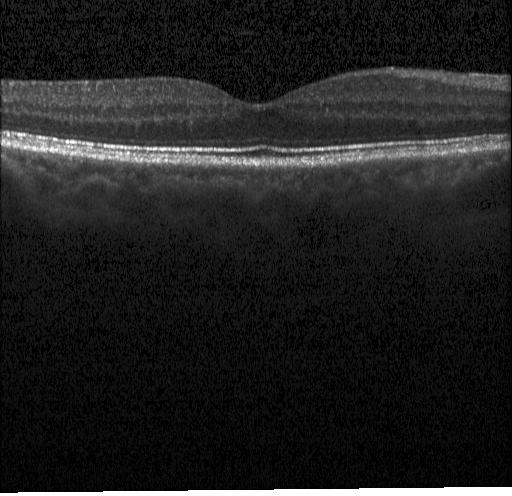
Optical coherence tomography scan.
OCT finding: neither CNV, DME, nor drusen.